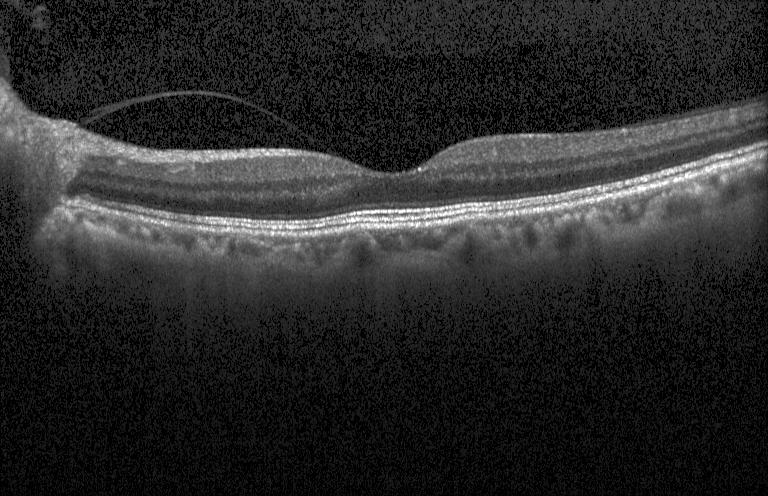

Heidelberg Spectralis; optical coherence tomography B-scan
Diagnosis: neither CNV, DME, nor drusen.